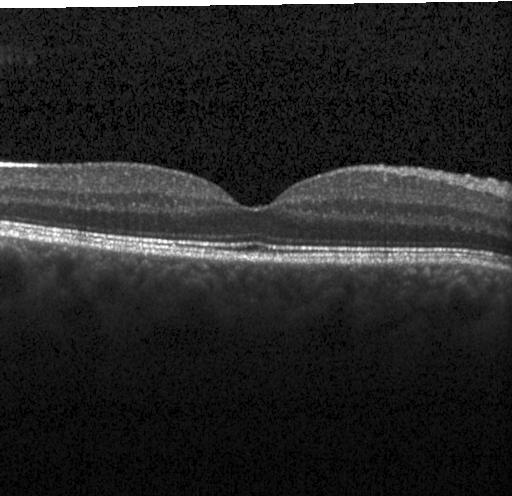 This B-scan demonstrates neither choroidal neovascularization, diabetic macular edema, nor drusen.